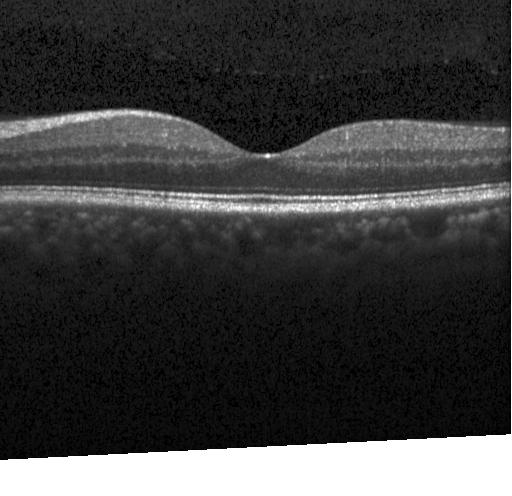

OCT line scan. Spectral-domain OCT. Fovea-centered.
The scan shows no CNV, no DME, and no drusen.